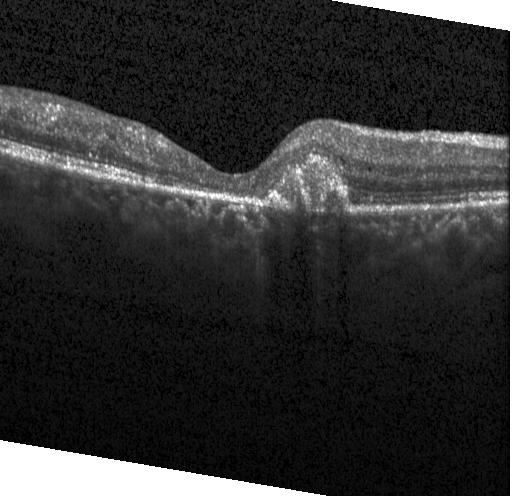
Through the macula, instrument: Heidelberg Spectralis, spectral-domain optical coherence tomography, retinal OCT B-scan.
Finding: a choroidal neovascular membrane.